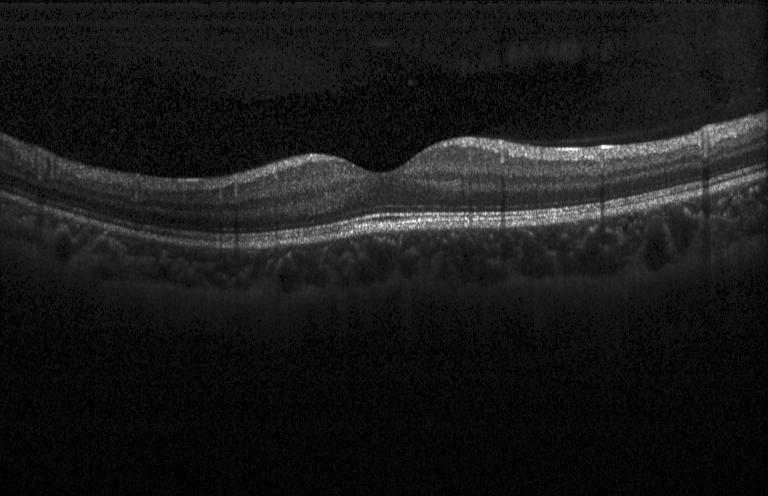 Optical coherence tomography scan · spectral-domain optical coherence tomography. Finding: neither CNV, DME, nor drusen.